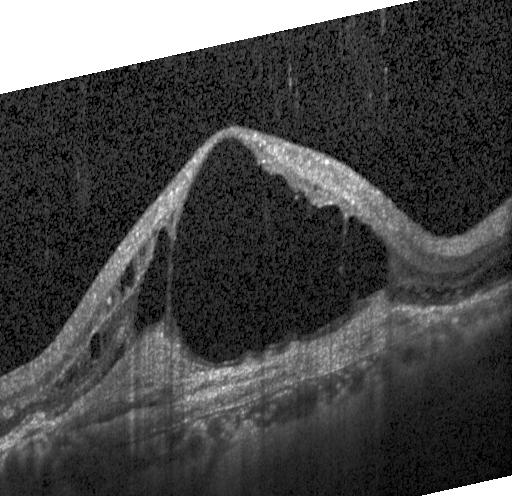
Spectral-domain OCT B-scan: choroidal neovascularization.